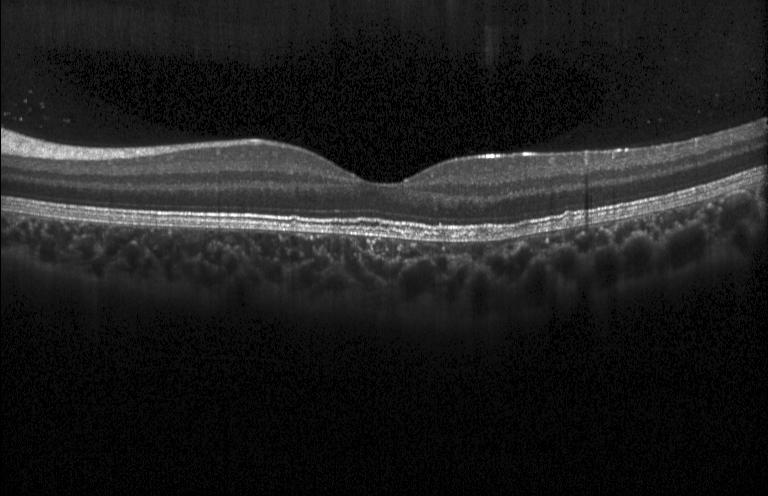

Optical coherence tomography B-scan — The scan shows no choroidal neovascularization, no diabetic macular edema, and no drusen.